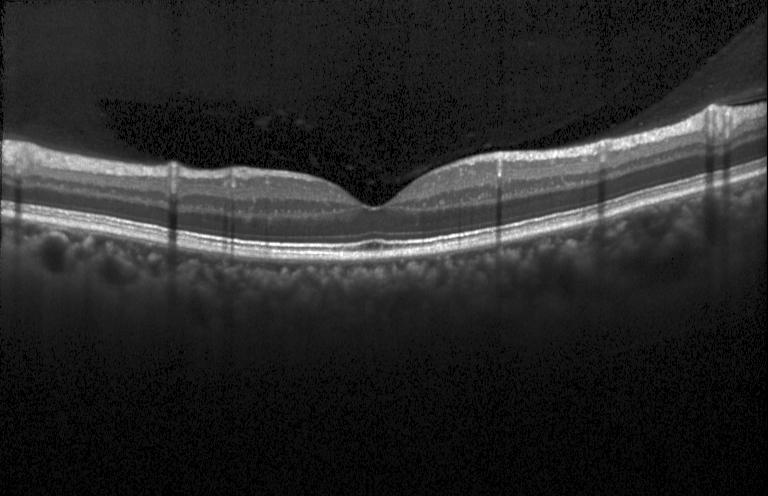

Assessment: no evidence of choroidal neovascularization, diabetic macular edema, or drusen.